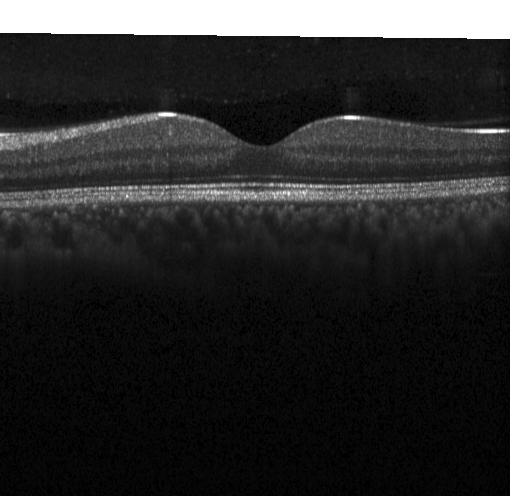

SD-OCT. Centered on the fovea. Retinal OCT B-scan.
The scan shows no choroidal neovascularization, no diabetic macular edema, and no drusen.